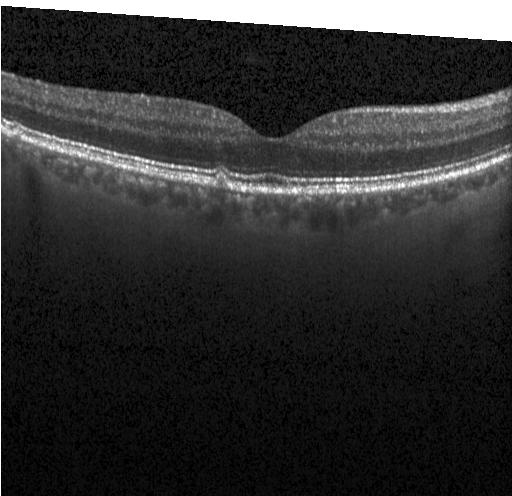 Dx: drusen.